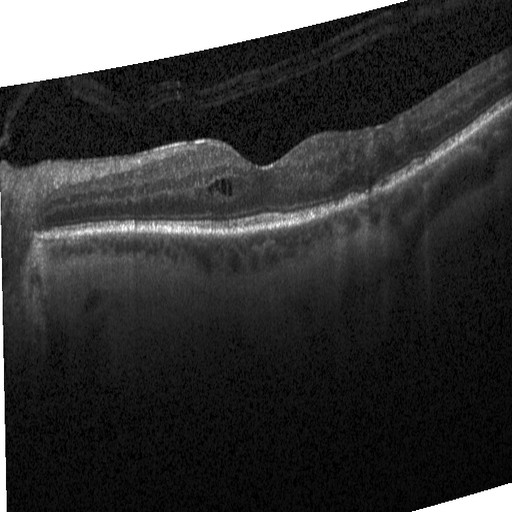 Optical coherence tomography B-scan
Finding: DME.